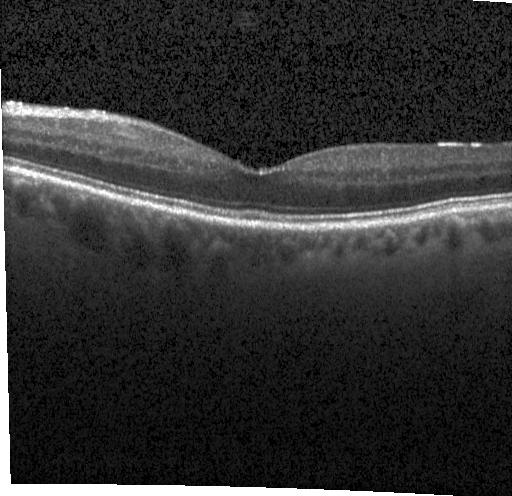 No choroidal neovascularization, diabetic macular edema, or drusen.